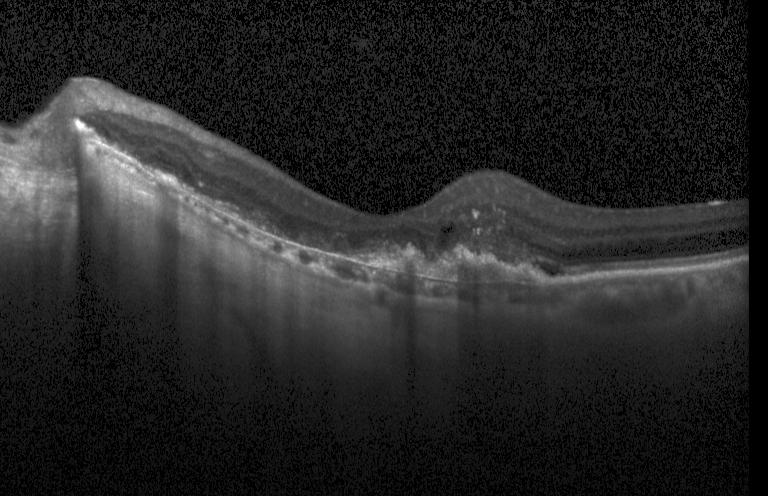
Retinal OCT B-scan; acquired on a Heidelberg Spectralis — Diagnosis: choroidal neovascularization (CNV).